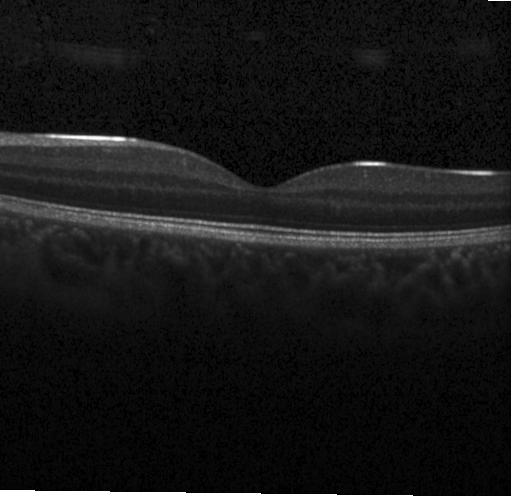
Macular OCT: no choroidal neovascularization, diabetic macular edema, or drusen.